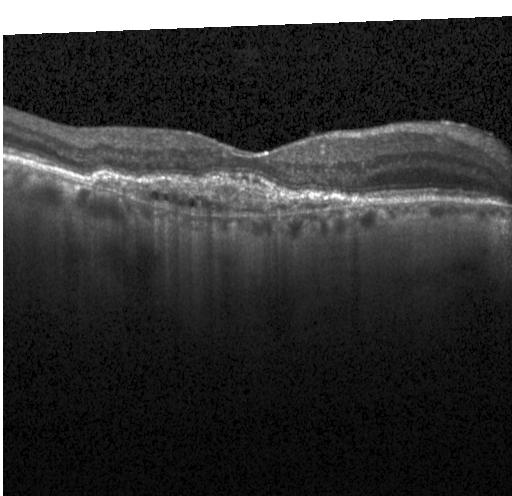
Choroidal neovascularization.